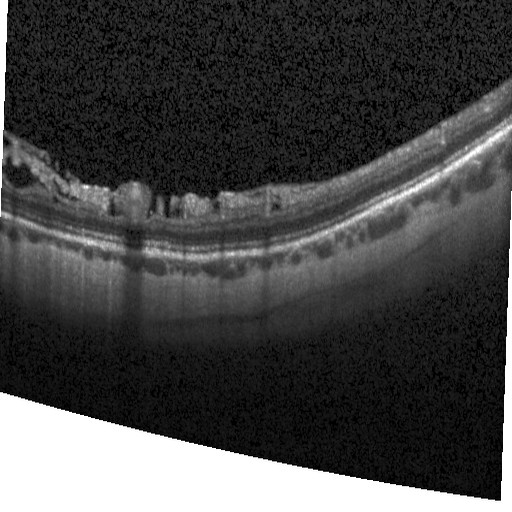 Retinal OCT cross-section, spectral-domain optical coherence tomography, Heidelberg Spectralis OCT system, fovea-centered.
Dx: diabetic macular edema.